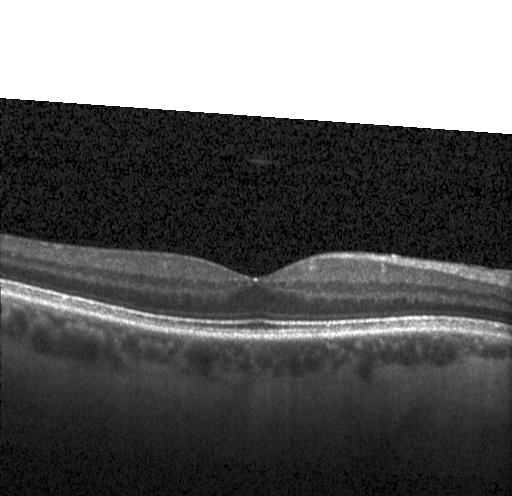

Retinal OCT cross-section showing no choroidal neovascularization, diabetic macular edema, or drusen.